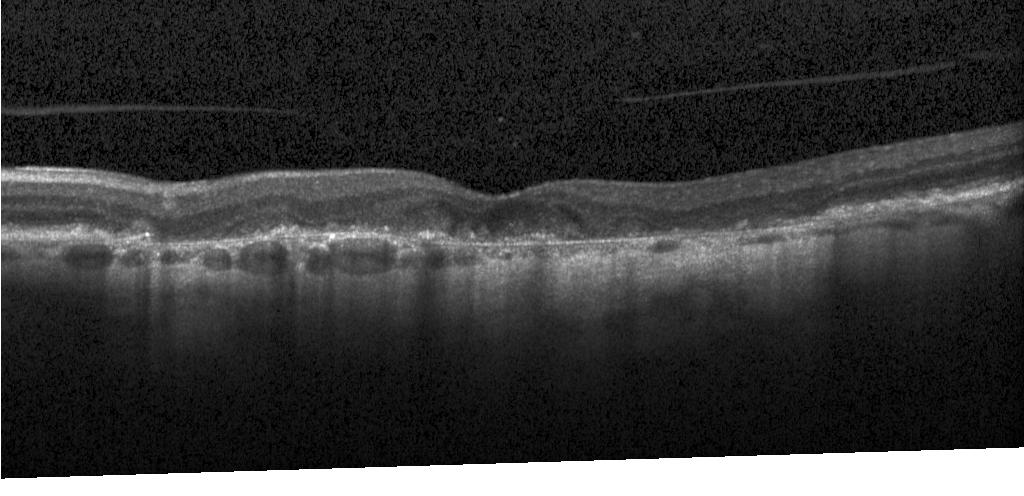
Retinal OCT B-scan. Spectral-domain optical coherence tomography.
Diagnosis: no evidence of choroidal neovascularization, diabetic macular edema, or drusen.